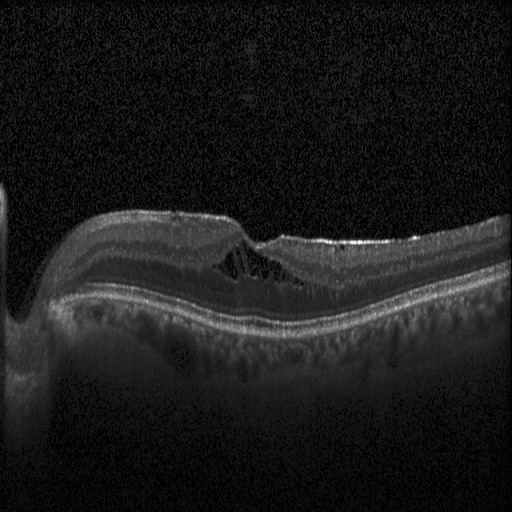
Diagnosis: diabetic macular edema (DME).